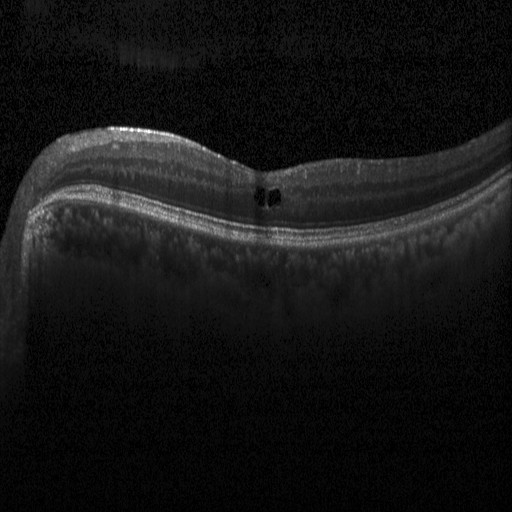
SD-OCT · Heidelberg Spectralis OCT system · retinal OCT B-scan.
The scan shows DME.